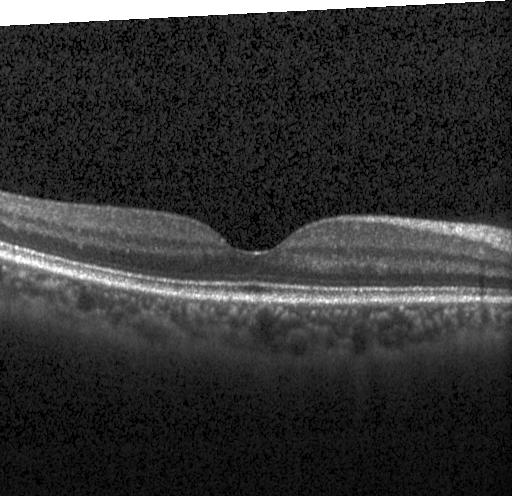

Finding: no evidence of CNV, DME, or drusen.